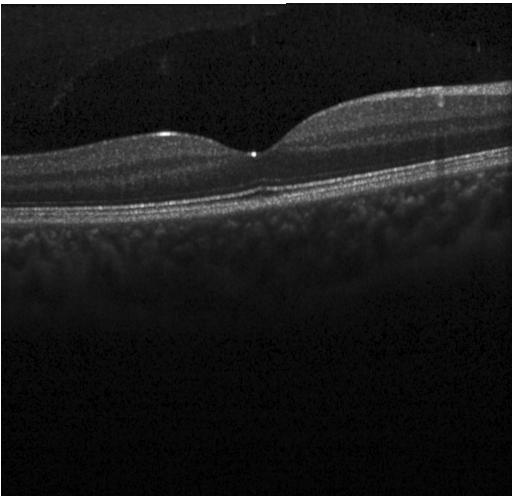 Retinal OCT cross-section; centered on the fovea; spectral-domain optical coherence tomography — Assessment: neither CNV, DME, nor drusen.